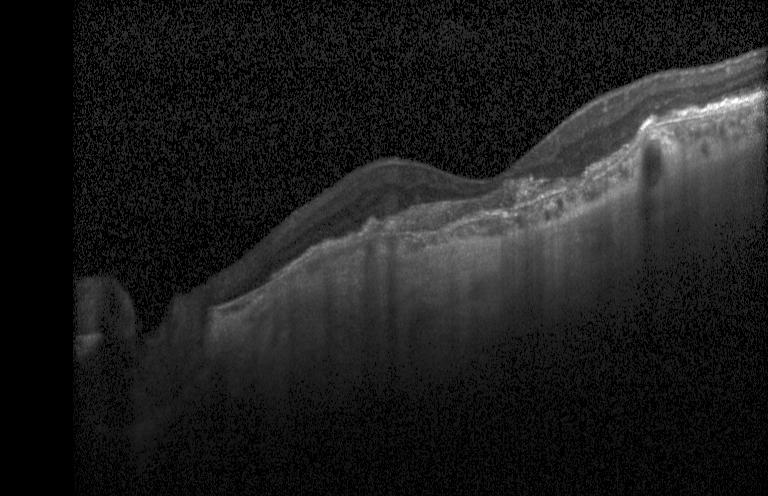 Acquired on a Heidelberg Spectralis. Retinal OCT B-scan. Horizontal scan through the fovea. Spectral-domain OCT. Diagnosis: a choroidal neovascular membrane.